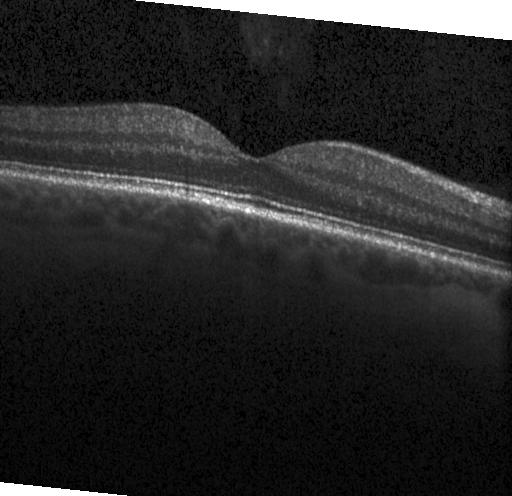 Diagnosis: neither CNV, DME, nor drusen.